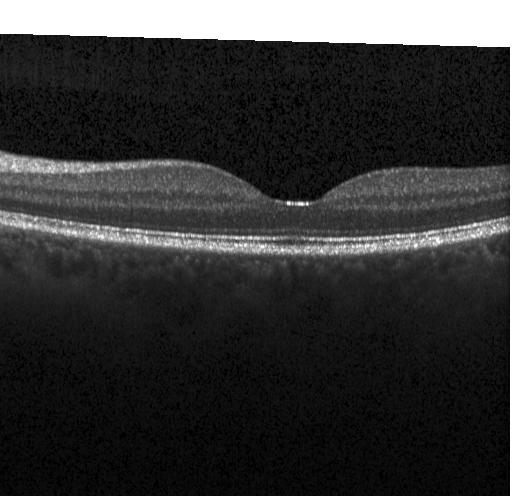
This B-scan demonstrates no CNV, no DME, and no drusen.